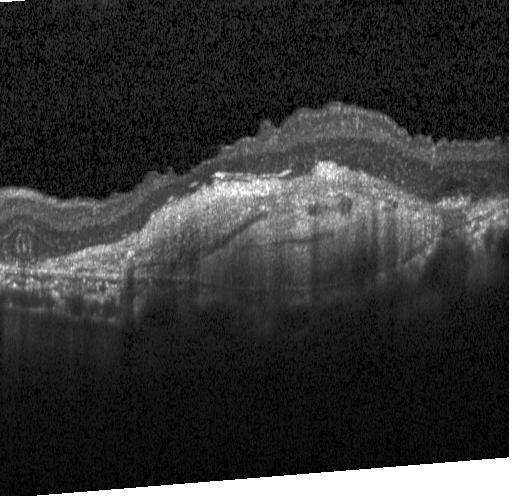

Finding: a choroidal neovascular membrane.